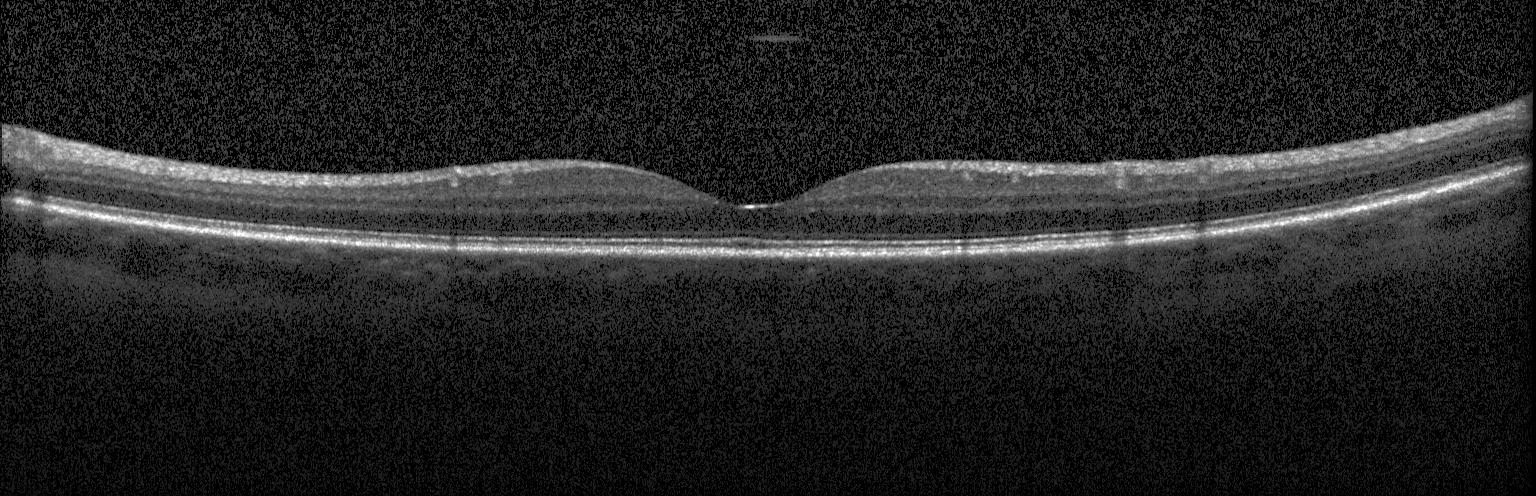

Optical coherence tomography scan.
Assessment: no choroidal neovascularization, no diabetic macular edema, and no drusen.